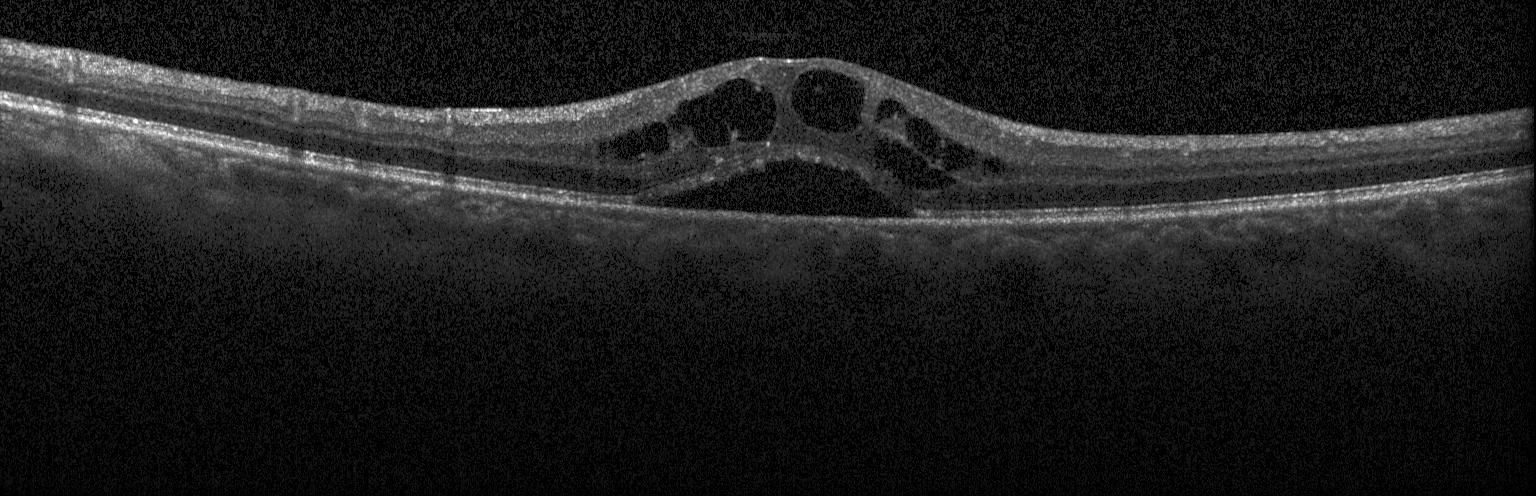
Heidelberg Spectralis, OCT line scan, SD-OCT, centered on the fovea
Macular OCT: diabetic macular edema.